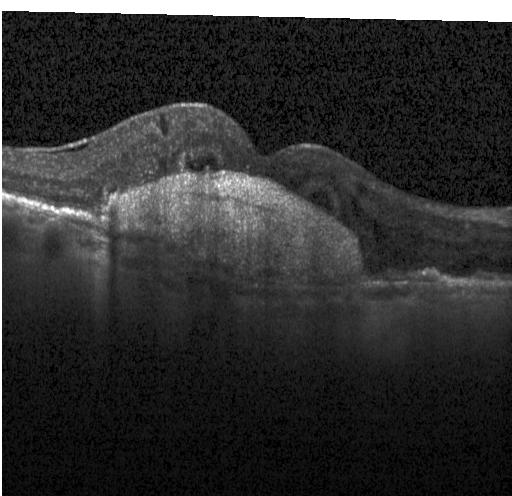
Retinal OCT cross-section; instrument: Heidelberg Spectralis — A choroidal neovascular membrane.